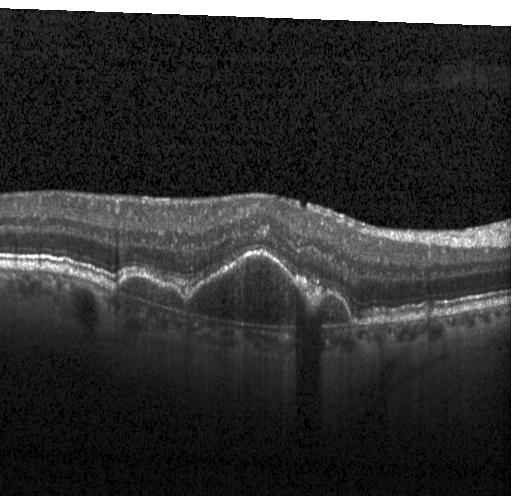
Impression: a choroidal neovascular membrane.